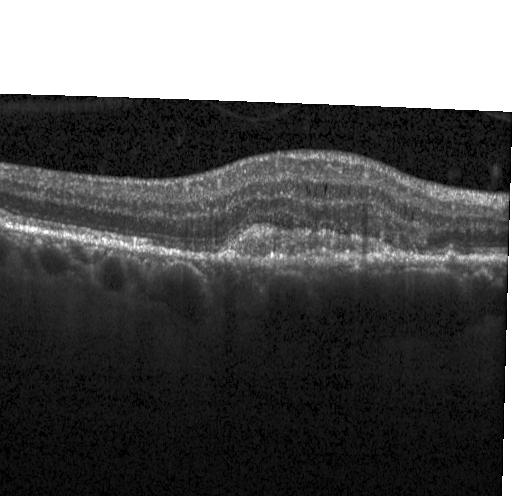
Dx: CNV.